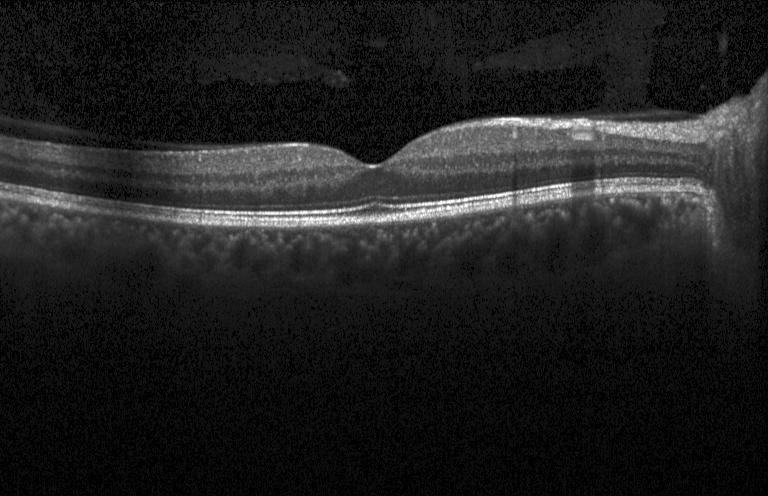 Optical coherence tomography B-scan. SD-OCT
Diagnosis: no CNV, DME, or drusen.